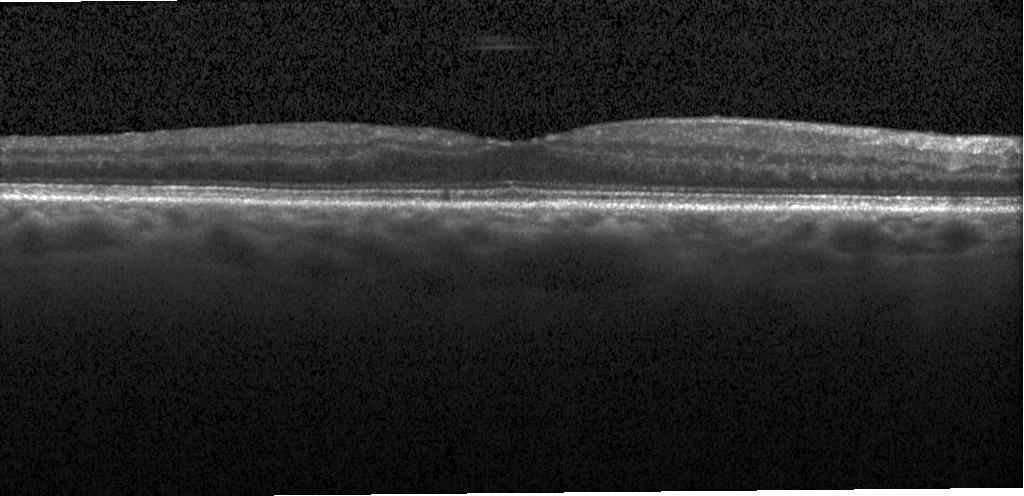

Diagnosis: neither choroidal neovascularization, diabetic macular edema, nor drusen.